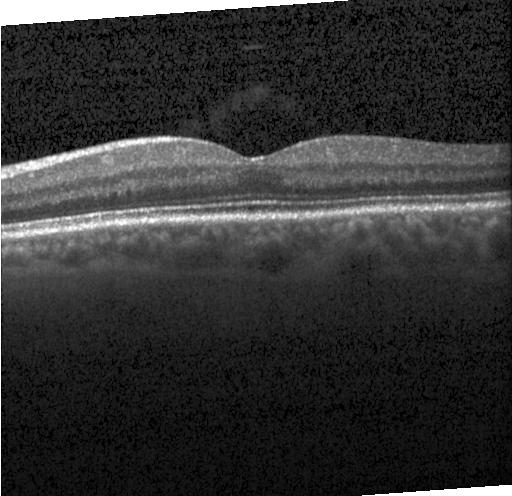 OCT line scan
This B-scan demonstrates neither CNV, DME, nor drusen.